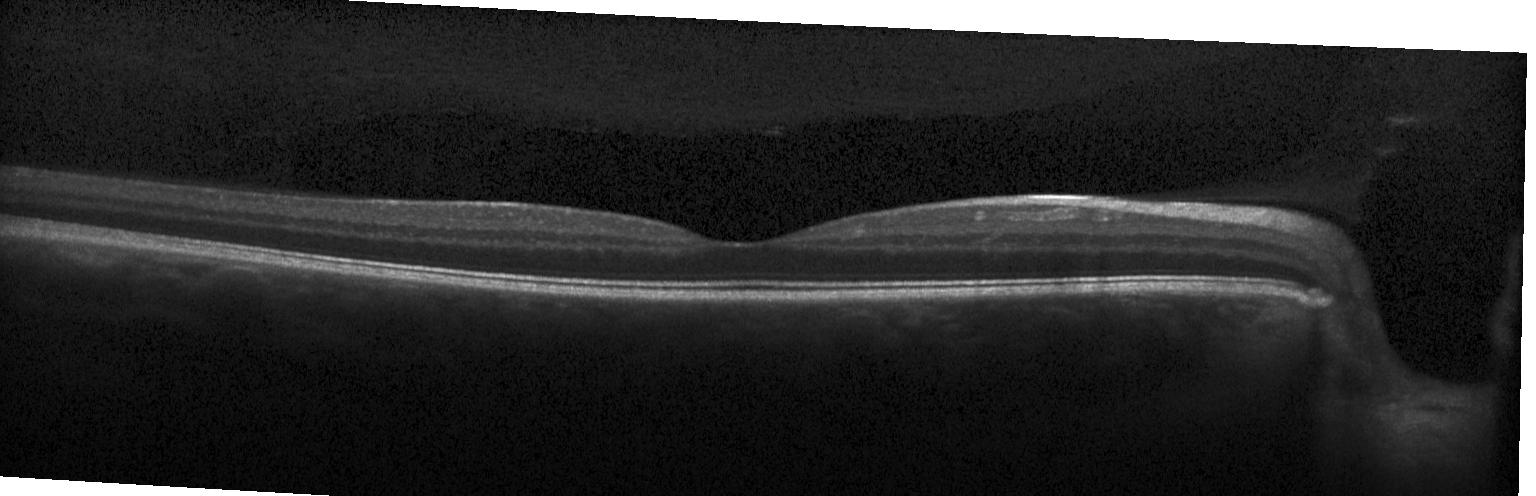

Diagnosis: no evidence of CNV, DME, or drusen.